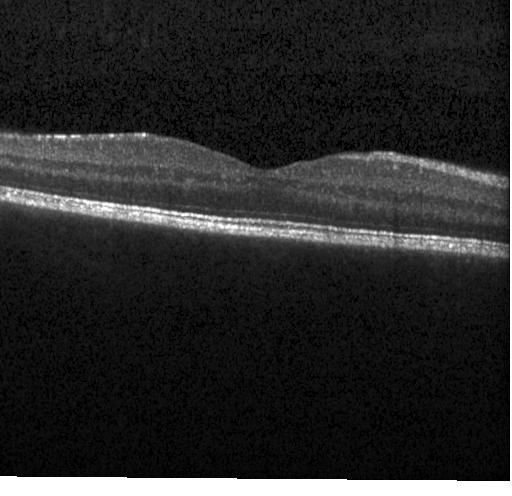 Horizontal scan through the fovea · retinal OCT B-scan · Heidelberg Spectralis. OCT finding: no choroidal neovascularization, no diabetic macular edema, and no drusen.